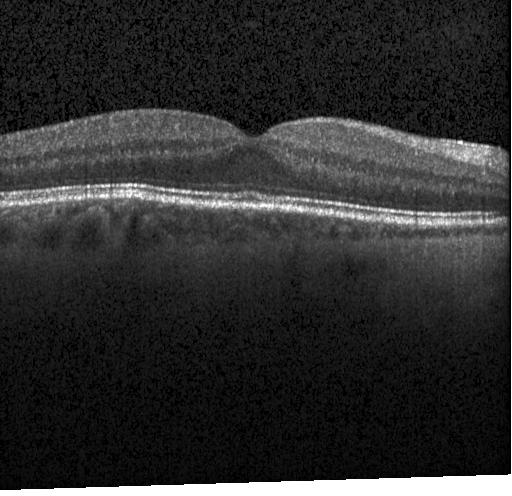

This B-scan demonstrates no CNV, no DME, and no drusen.